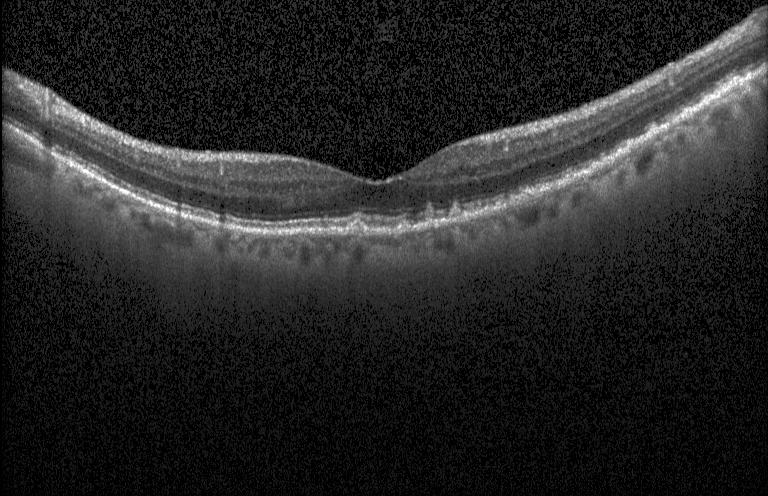
Optical coherence tomography scan. Fovea-centered
Macular OCT: multiple drusen.